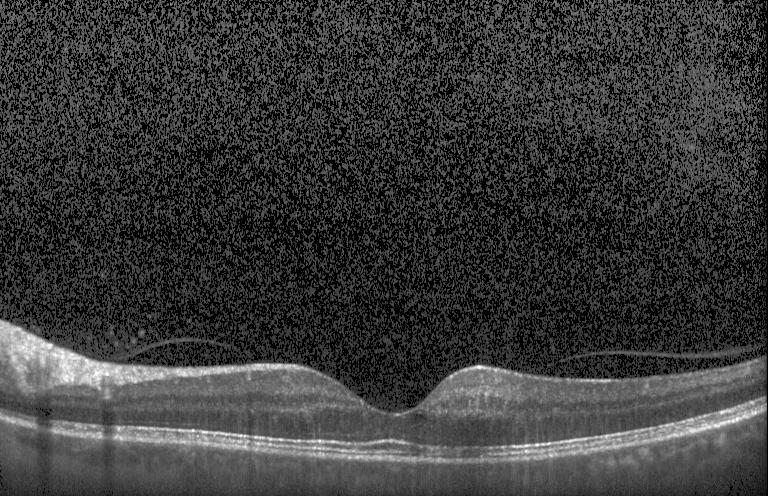 SD-OCT. Horizontal scan through the fovea. Heidelberg Spectralis OCT system. OCT line scan.
Dx: no CNV, no DME, and no drusen.